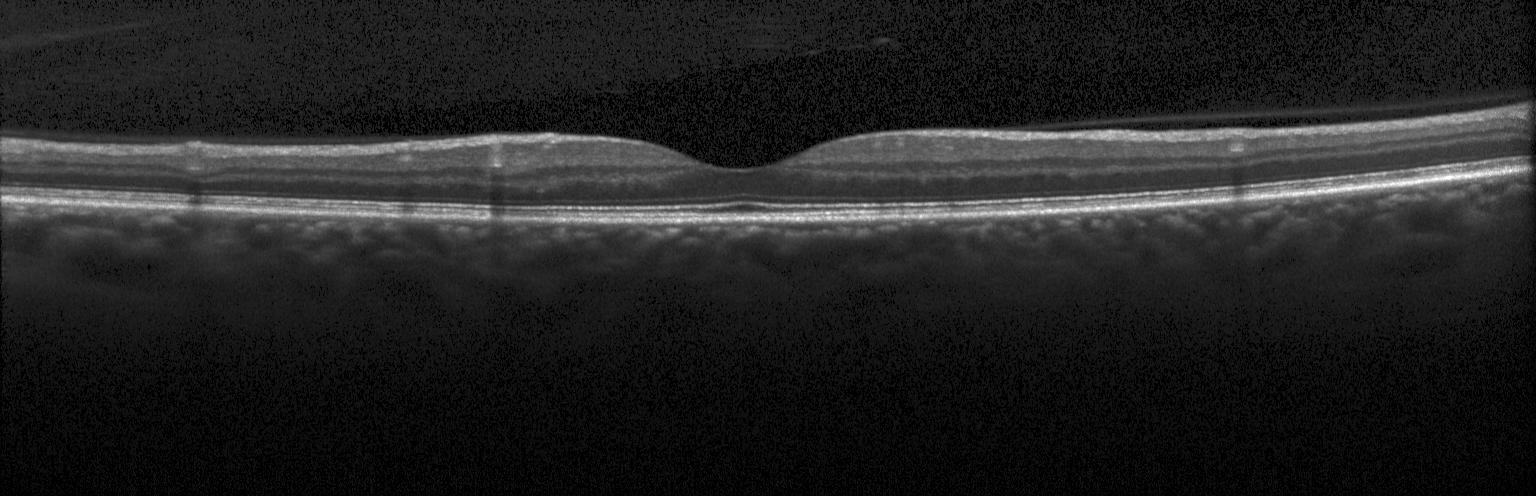

Optical coherence tomography B-scan
Finding: no CNV, DME, or drusen.